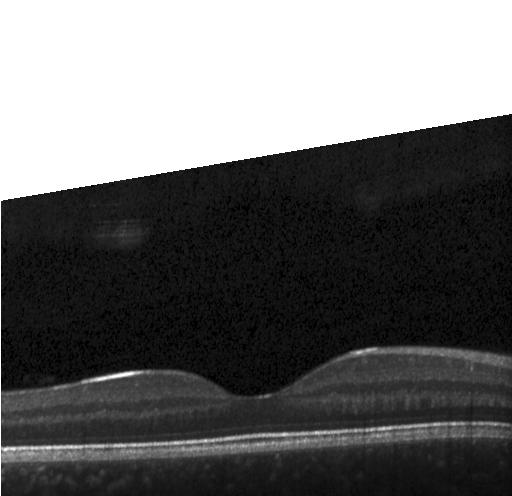

Fovea-centered · optical coherence tomography B-scan · spectral-domain optical coherence tomography · instrument: Heidelberg Spectralis.
Finding: no choroidal neovascularization, no diabetic macular edema, and no drusen.